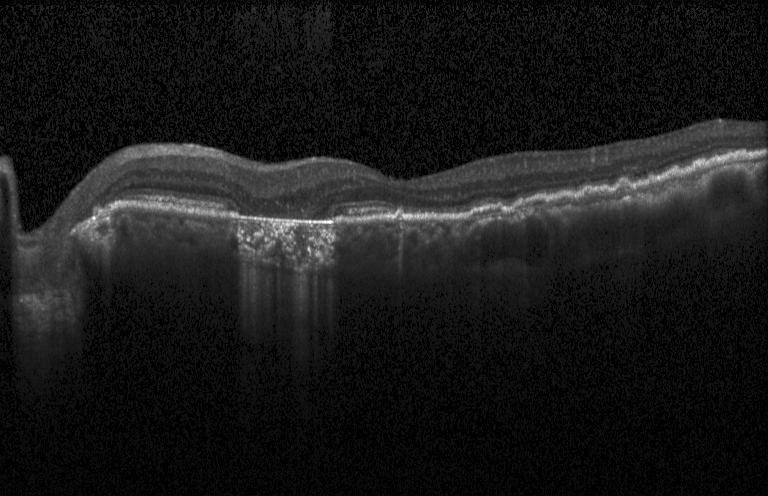

Optical coherence tomography scan, spectral-domain OCT. The scan shows CNV.